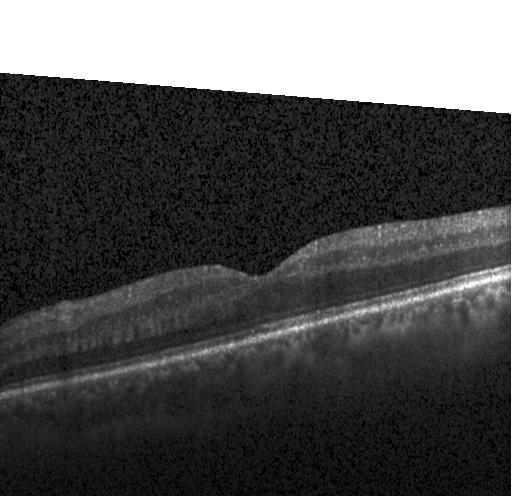
Macular OCT demonstrating no choroidal neovascularization, no diabetic macular edema, and no drusen.